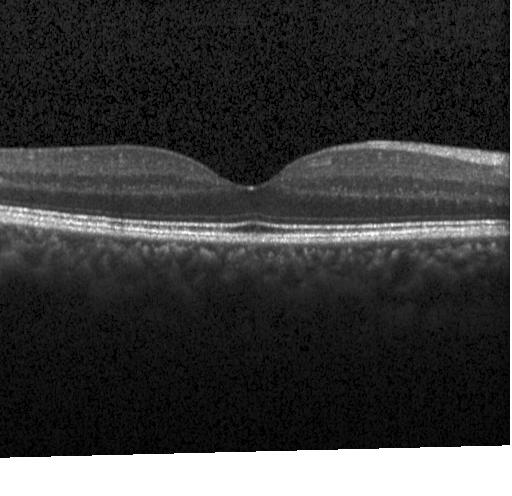 OCT finding: no CNV, no DME, and no drusen.